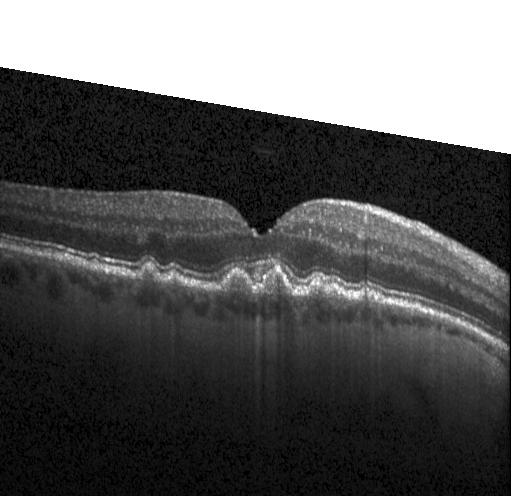
Optical coherence tomography scan — Impression: drusen.